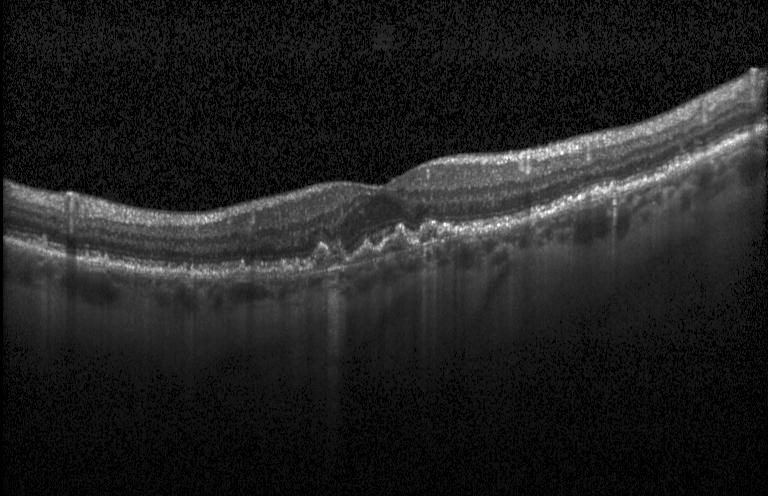

Retinal OCT B-scan. Spectral-domain OCT. Through the macula. Acquired on a Heidelberg Spectralis — OCT finding: a choroidal neovascular membrane.